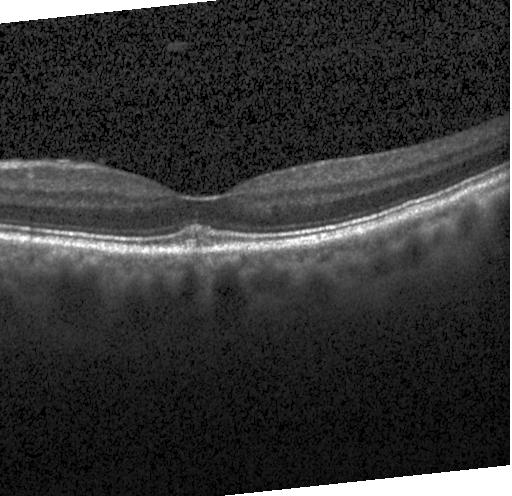 Retinal OCT B-scan. SD-OCT. Heidelberg Spectralis OCT system — Assessment: neither choroidal neovascularization, diabetic macular edema, nor drusen.